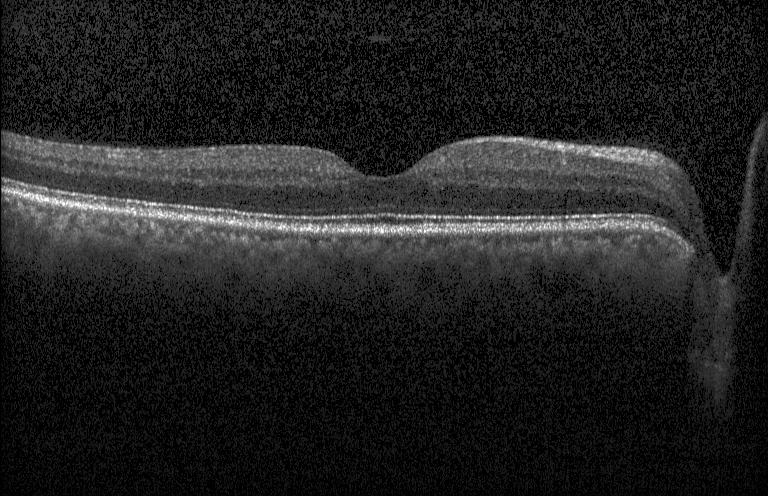
Macular OCT: no CNV, no DME, and no drusen.